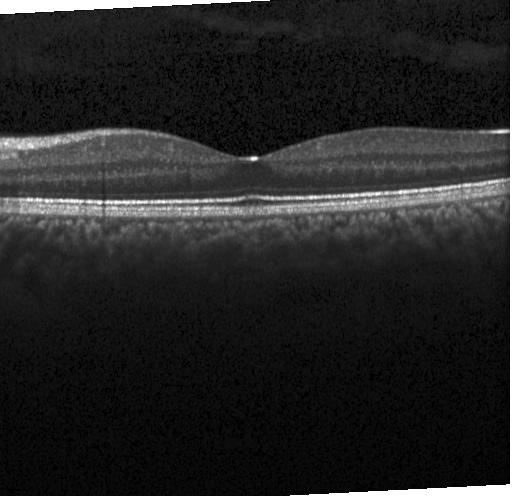 OCT scan showing no choroidal neovascularization, no diabetic macular edema, and no drusen.